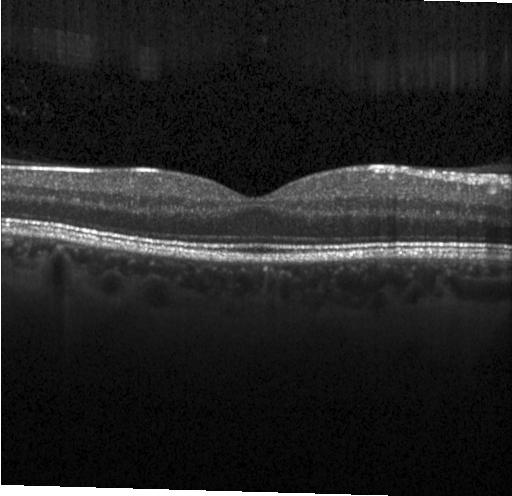 Dx: no CNV, DME, or drusen.